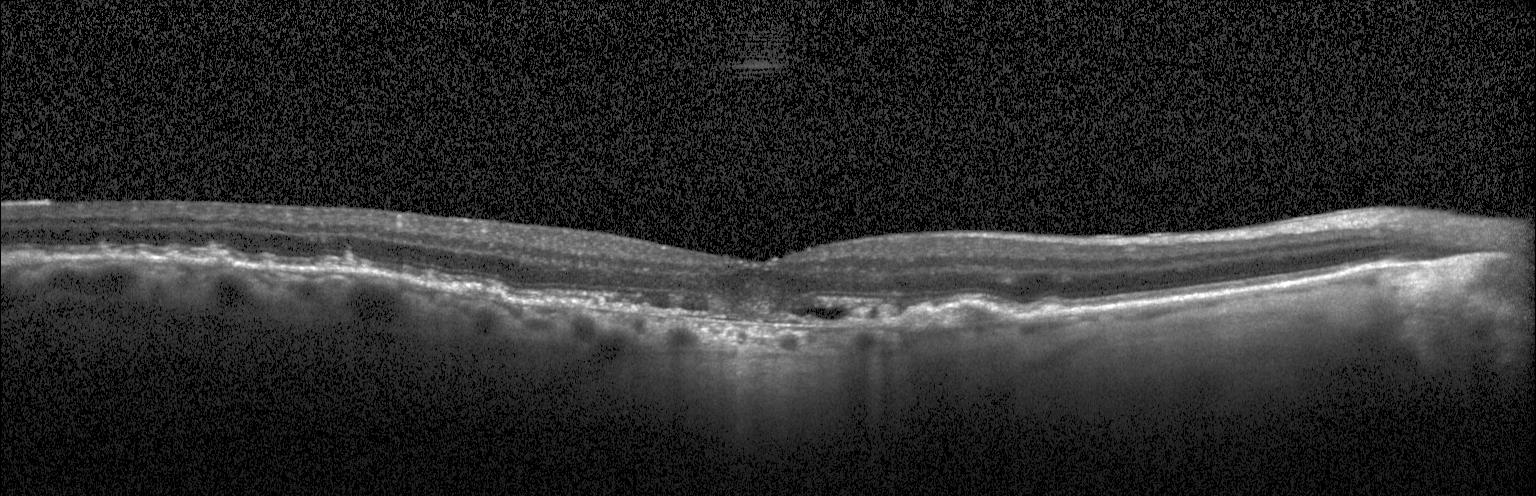
Dx: a choroidal neovascular membrane.